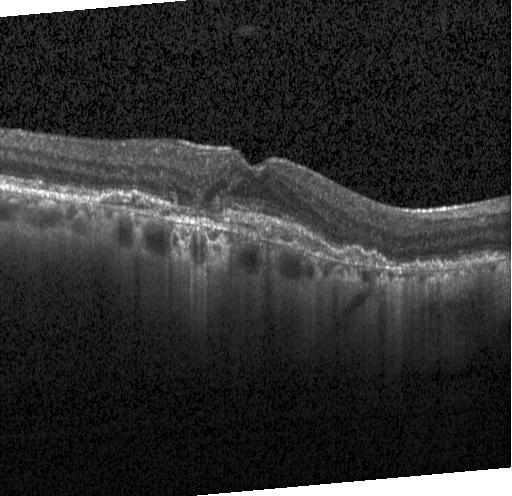
Retinal OCT B-scan. The scan shows choroidal neovascularization.